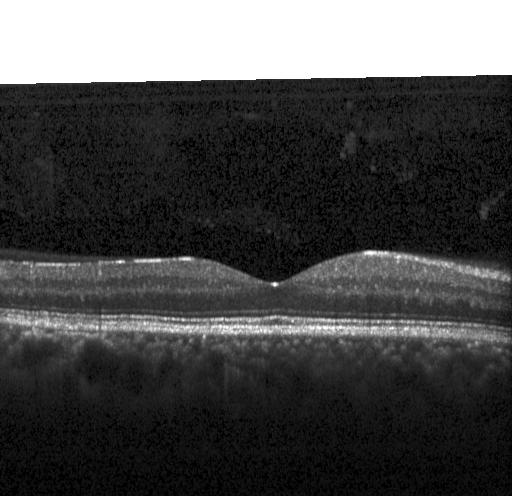 OCT B-scan.
Diagnosis: no choroidal neovascularization, no diabetic macular edema, and no drusen.